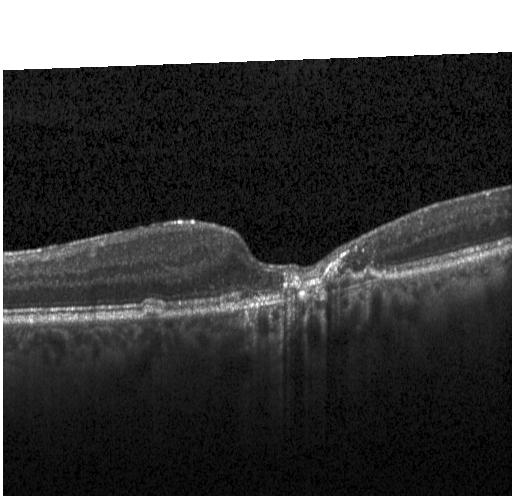 SD-OCT · OCT line scan
Impression: CNV.